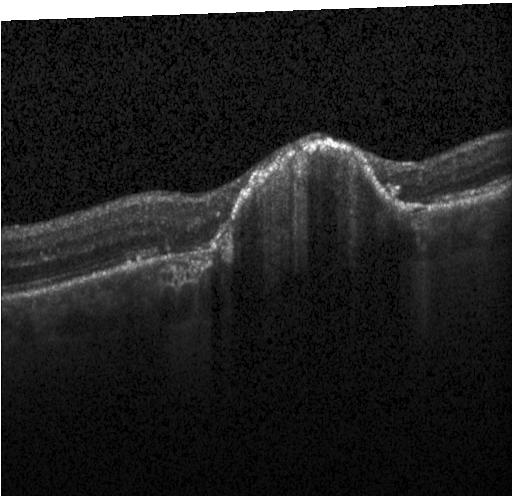

Finding: a choroidal neovascular membrane.